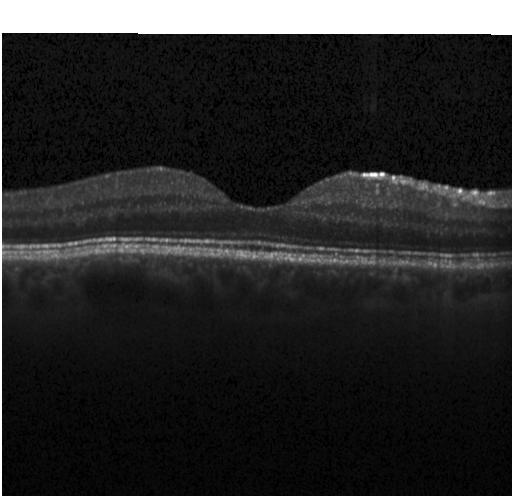
Optical coherence tomography B-scan; spectral-domain optical coherence tomography; acquired on a Heidelberg Spectralis
Assessment: no choroidal neovascularization, diabetic macular edema, or drusen.